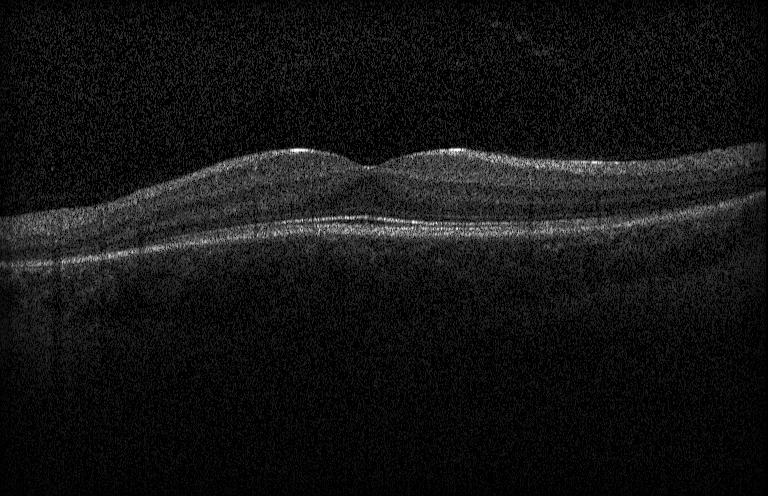

OCT line scan · instrument: Heidelberg Spectralis · spectral-domain OCT · macular scan — OCT finding: no choroidal neovascularization, no diabetic macular edema, and no drusen.